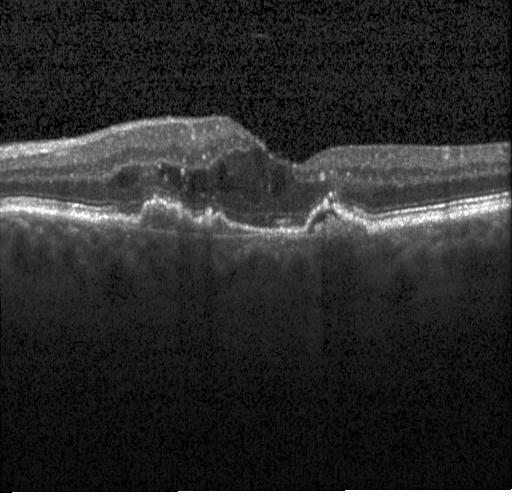 Fovea-centered. OCT B-scan. Spectral-domain optical coherence tomography — Impression: CNV.